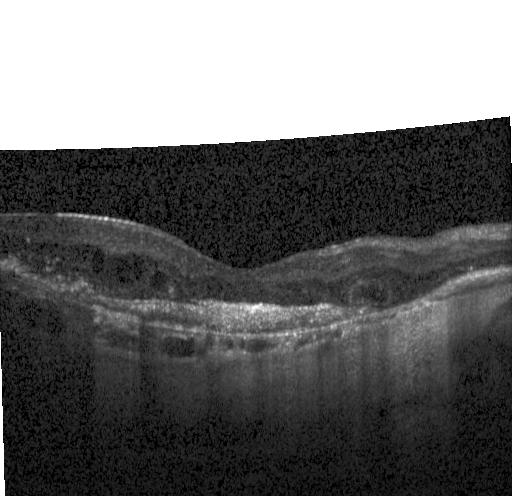
OCT B-scan, SD-OCT. Assessment: choroidal neovascularization (CNV).